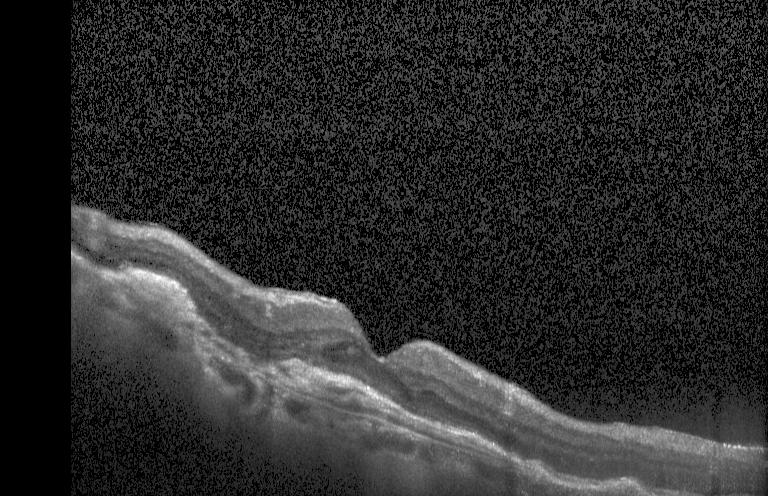 Heidelberg Spectralis · retinal OCT cross-section · spectral-domain OCT.
Dx: choroidal neovascularization (CNV).